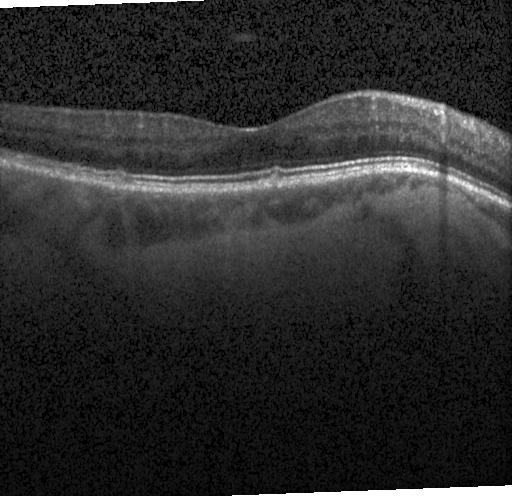 OCT finding: sub-RPE drusenoid deposits.